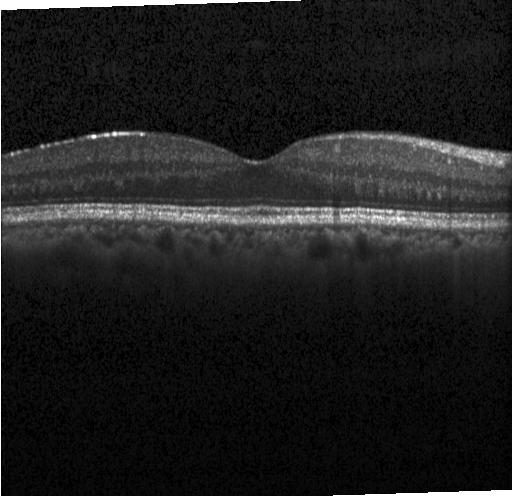
OCT line scan. Dx: no evidence of CNV, DME, or drusen.